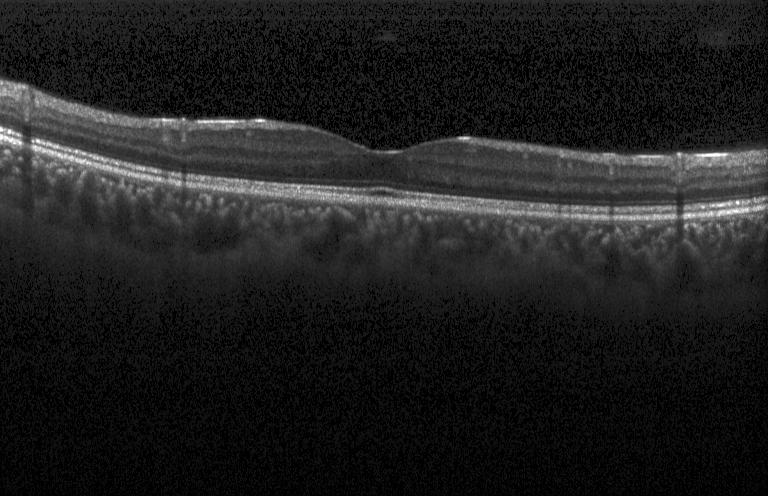
Dx: no CNV, no DME, and no drusen.